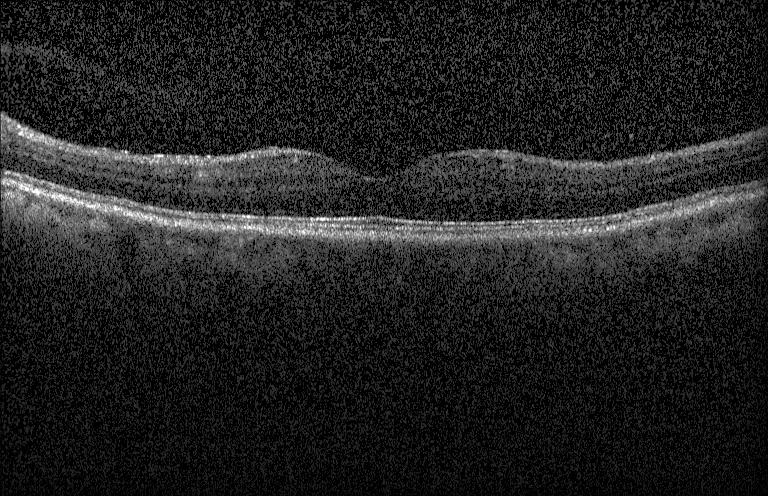
OCT B-scan showing neither CNV, DME, nor drusen.